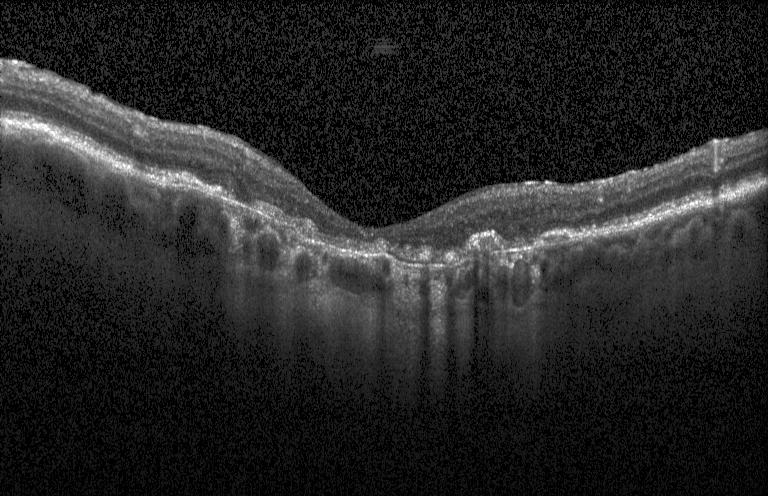 Optical coherence tomography B-scan · macular scan. Finding: a choroidal neovascular membrane.